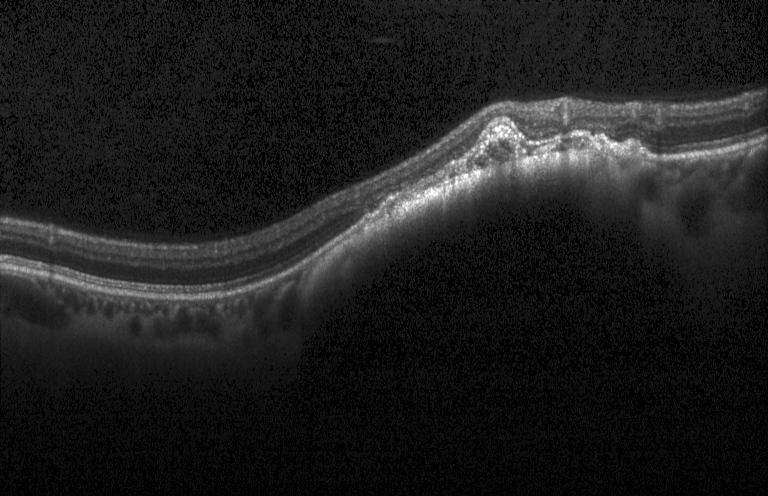
Spectral-domain OCT B-scan: choroidal neovascularization.